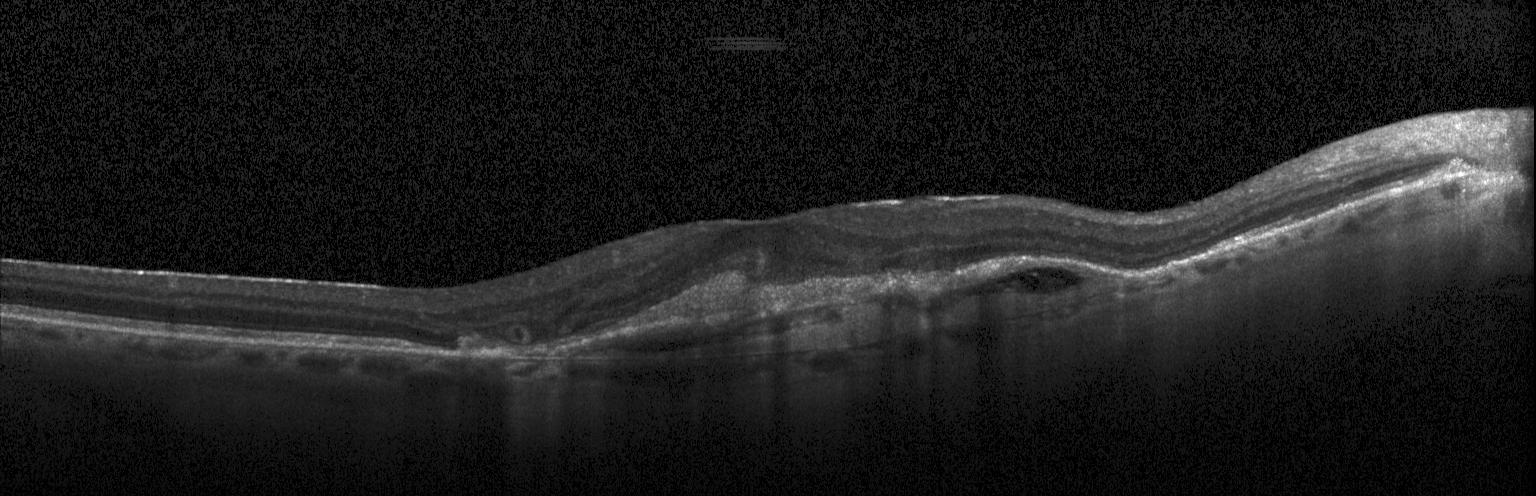 Spectral-domain optical coherence tomography. Optical coherence tomography scan. Acquired on a Heidelberg Spectralis
A choroidal neovascular membrane.